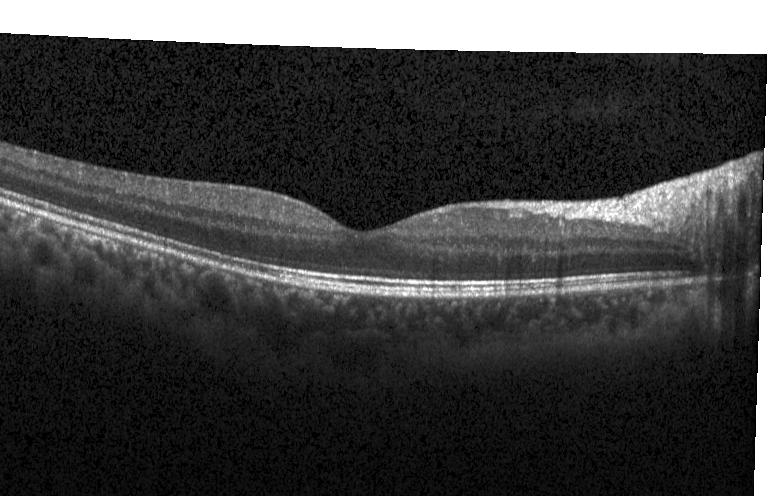
Retinal OCT B-scan, SD-OCT, fovea-centered, Heidelberg Spectralis OCT system. Impression: no choroidal neovascularization, diabetic macular edema, or drusen.